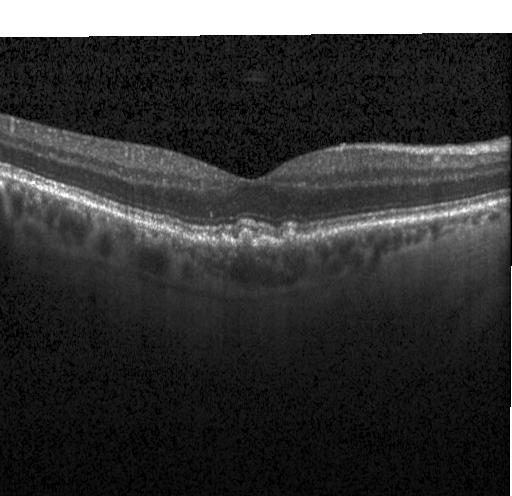

Diagnosis: multiple drusen.